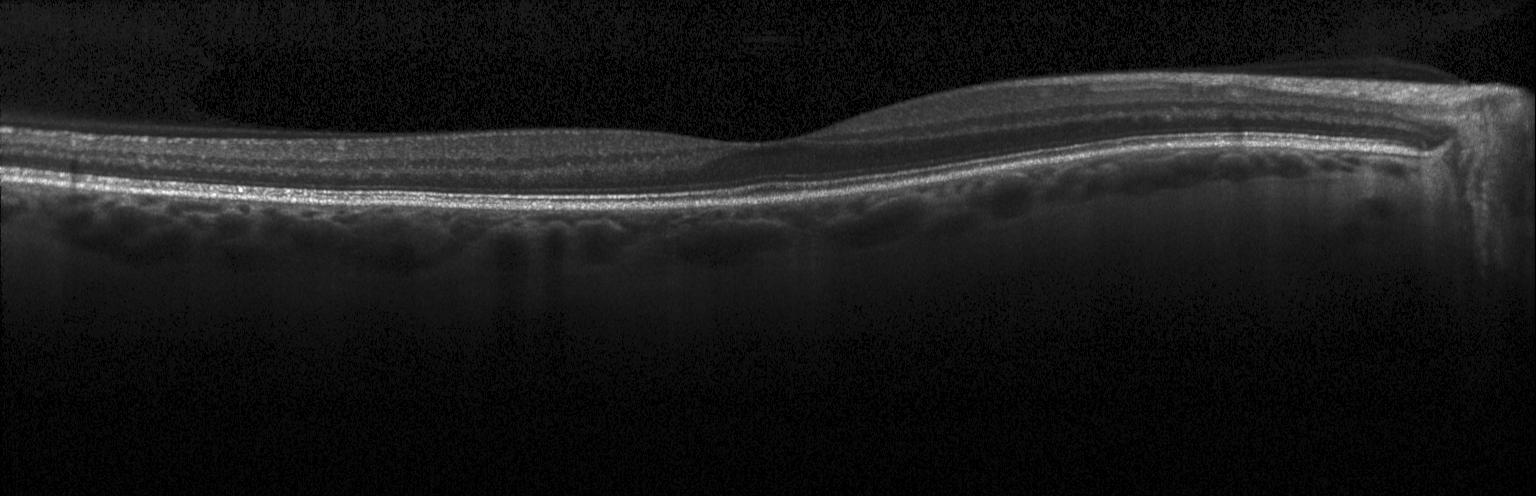
The scan shows no evidence of choroidal neovascularization, diabetic macular edema, or drusen.